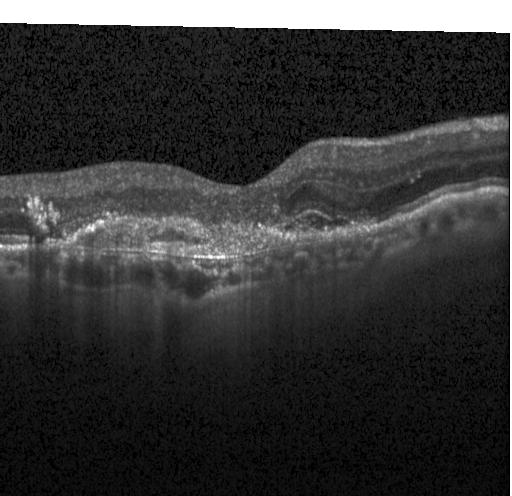 SD-OCT · Heidelberg Spectralis · fovea-centered · retinal OCT B-scan. Diagnosis: CNV.